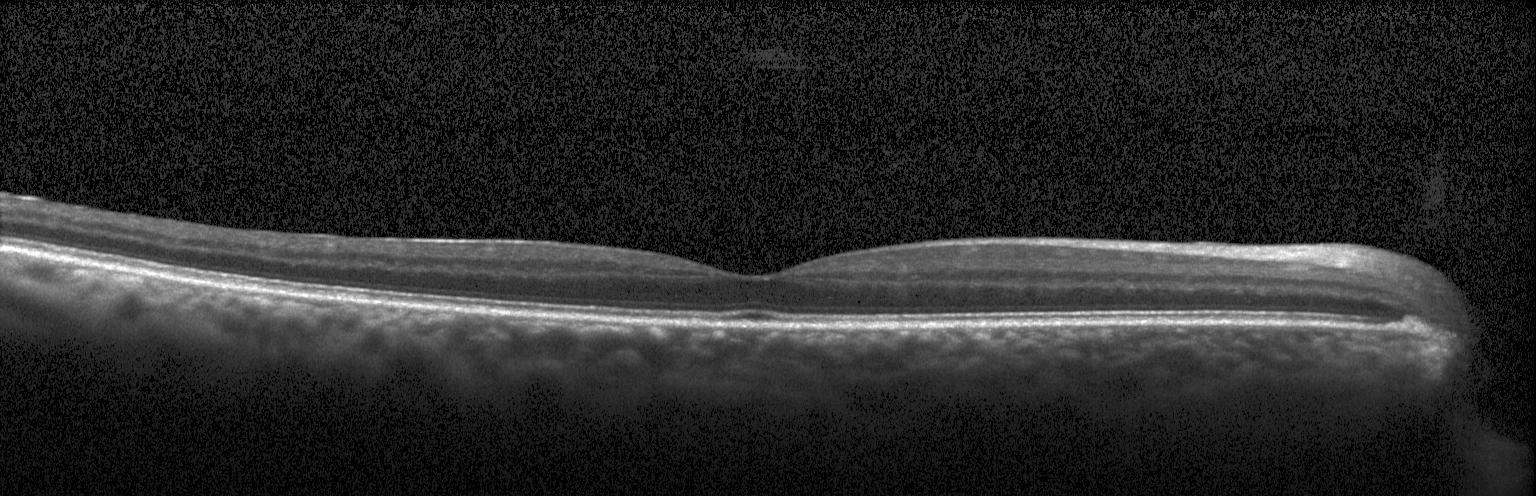 Dx: no CNV, DME, or drusen.